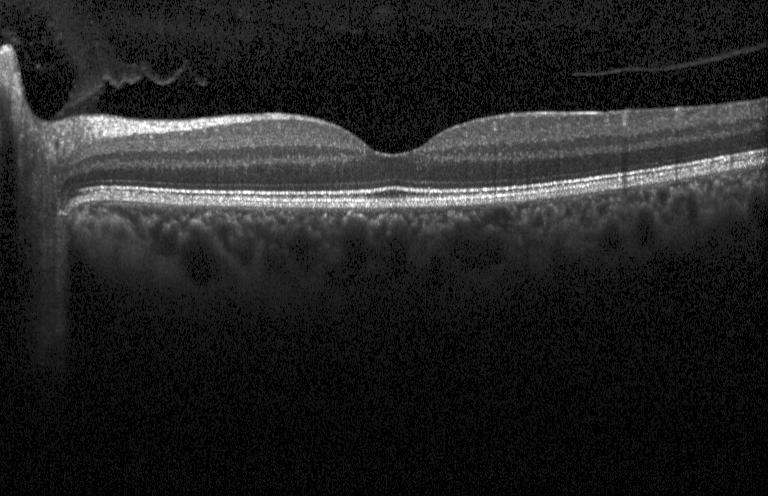

Macular OCT: no evidence of choroidal neovascularization, diabetic macular edema, or drusen.